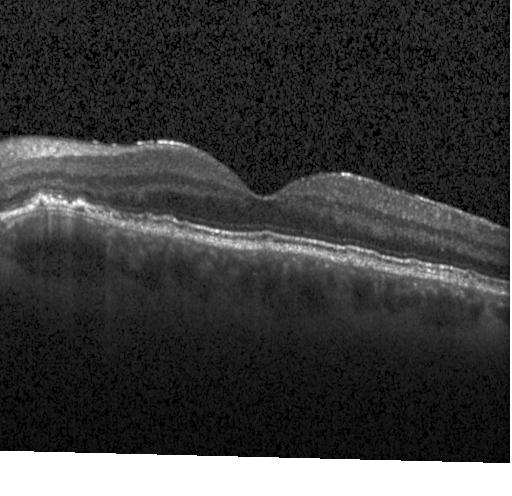
Impression: drusen.